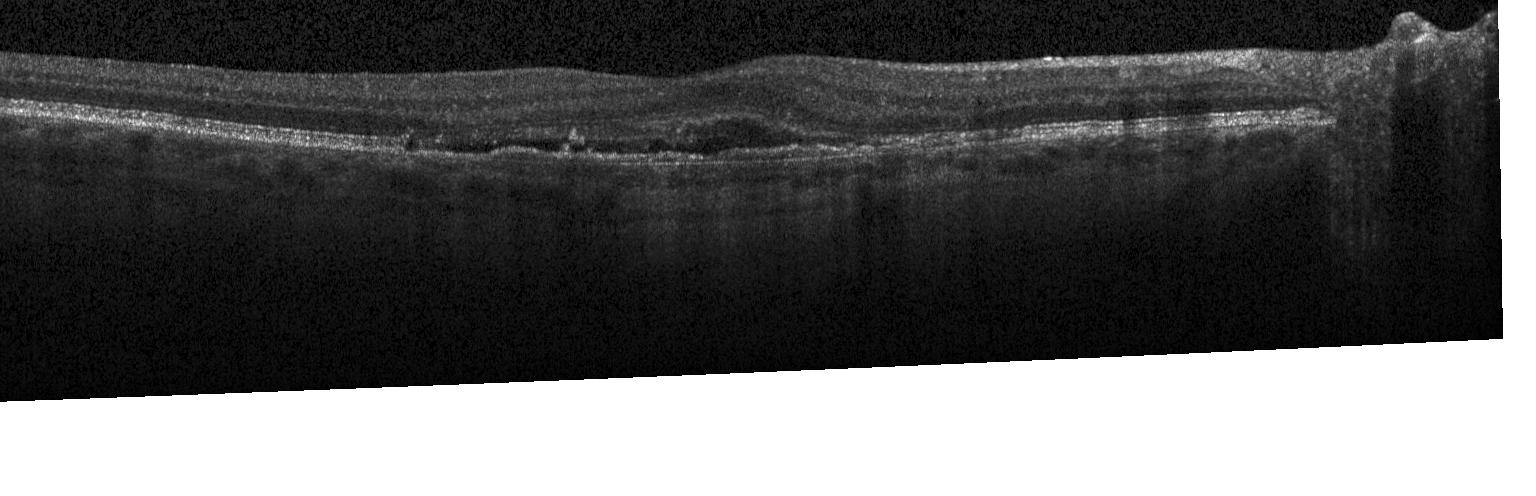
Spectral-domain OCT. Macular scan. Optical coherence tomography scan. Acquired on a Heidelberg Spectralis — Impression: a choroidal neovascular membrane.